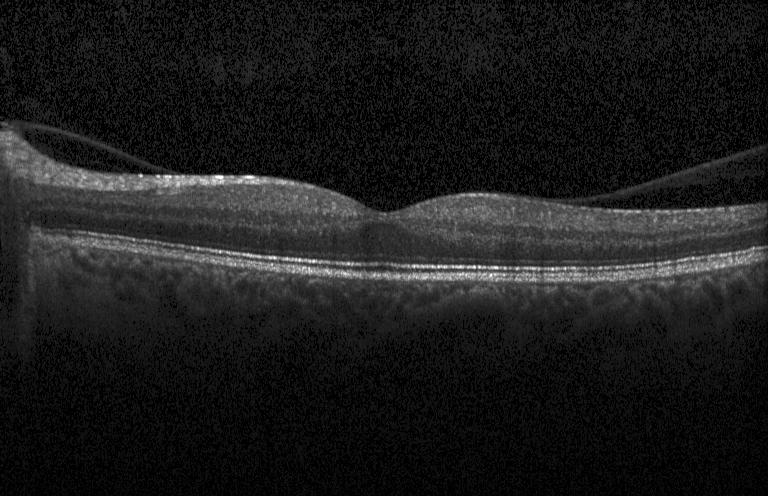 No choroidal neovascularization, no diabetic macular edema, and no drusen.